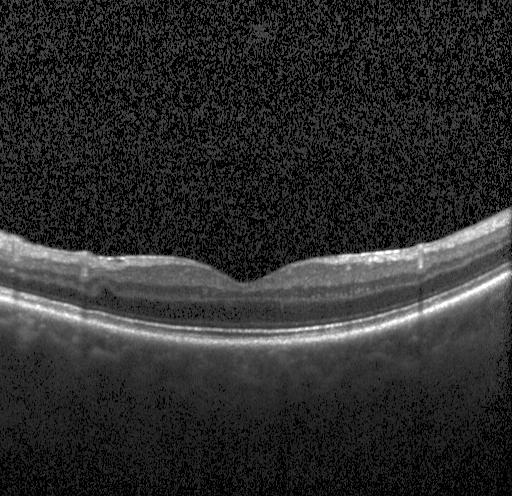

Through the macula; retinal OCT B-scan
Impression: no choroidal neovascularization, diabetic macular edema, or drusen.